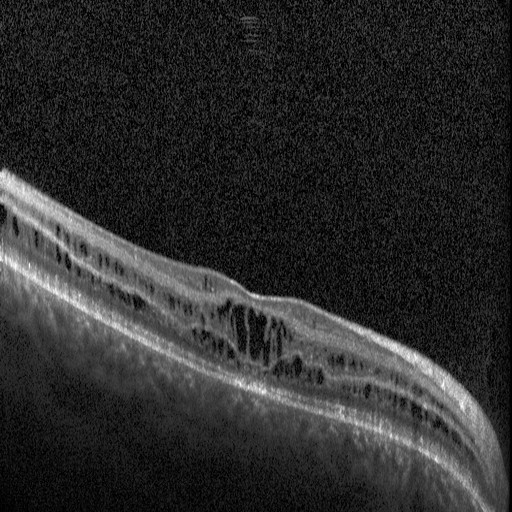

Finding: diabetic macular edema (DME).